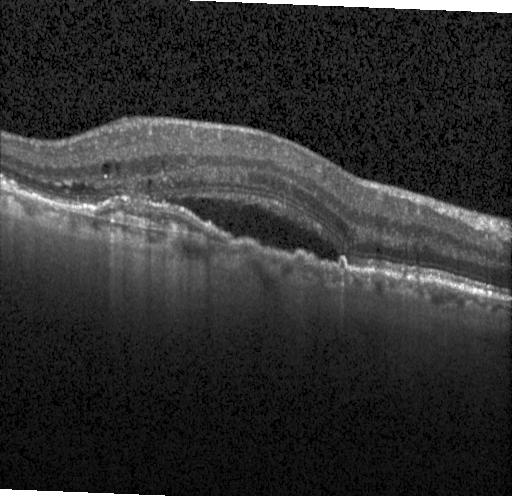

OCT line scan, through the macula — A choroidal neovascular membrane.